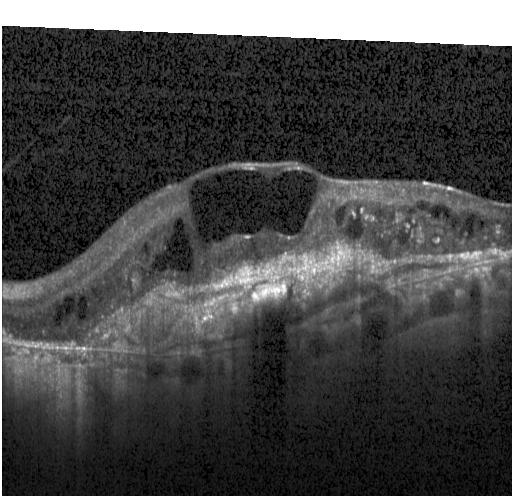

Macular OCT demonstrating choroidal neovascularization (CNV).